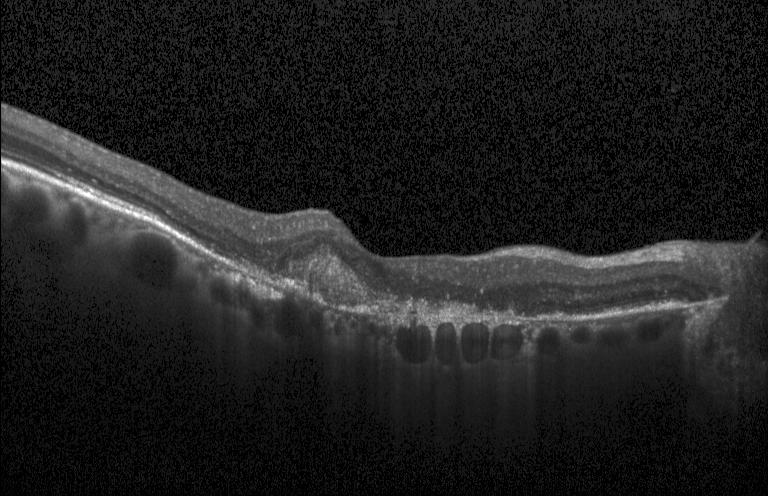
Spectral-domain OCT B-scan: a choroidal neovascular membrane.